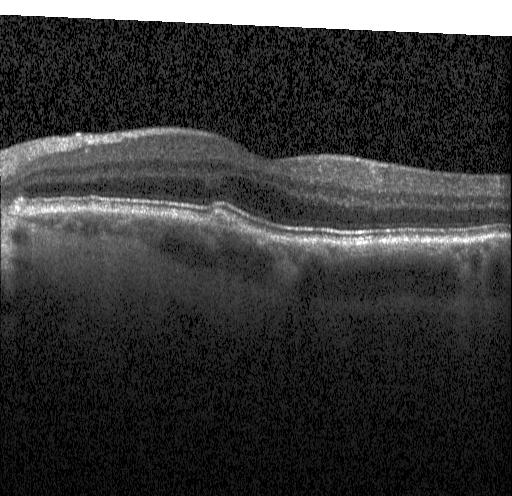
Dx: drusen.